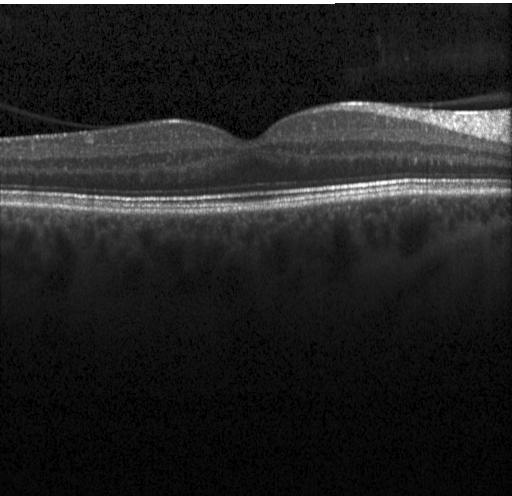
Macular scan, acquired on a Heidelberg Spectralis, SD-OCT, retinal OCT B-scan — OCT finding: neither choroidal neovascularization, diabetic macular edema, nor drusen.